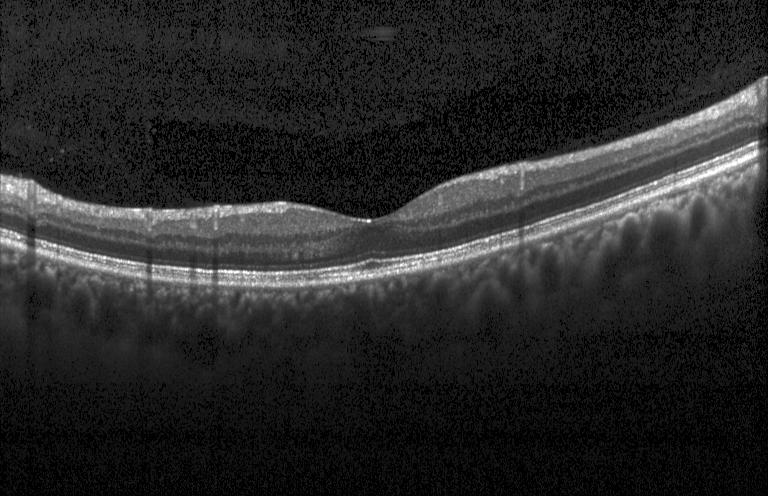

Retinal OCT cross-section — Dx: no evidence of CNV, DME, or drusen.